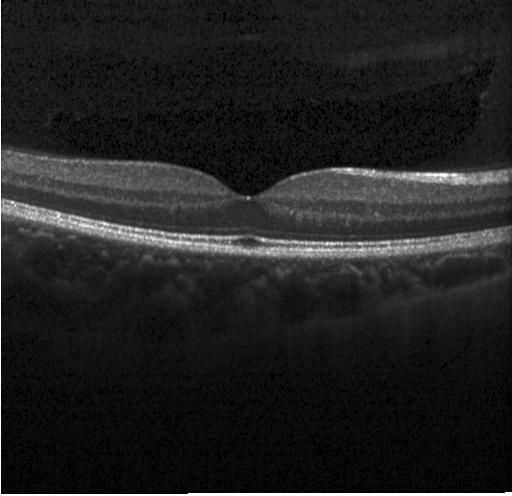

Heidelberg Spectralis OCT system · OCT line scan · spectral-domain OCT — Impression: no CNV, no DME, and no drusen.